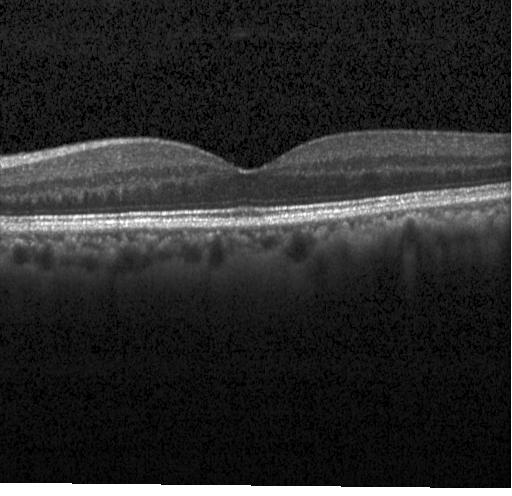
Macular scan. Heidelberg Spectralis. OCT line scan — Macular OCT: no choroidal neovascularization, no diabetic macular edema, and no drusen.